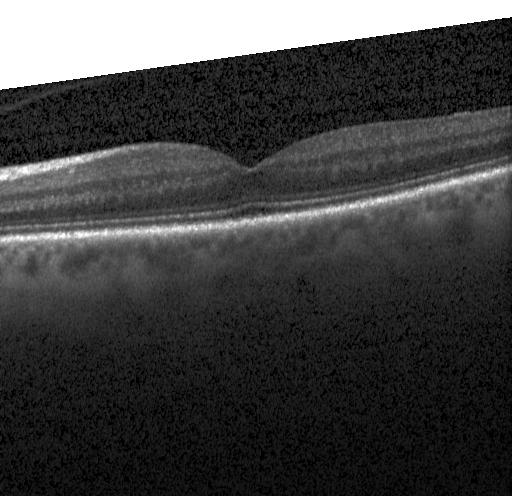
Dx: no evidence of CNV, DME, or drusen.